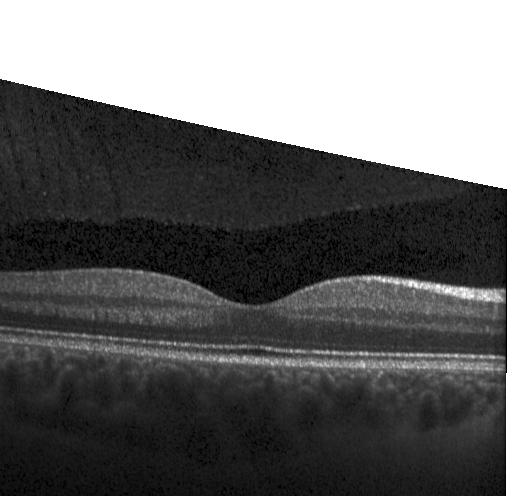

Fovea-centered. OCT B-scan. SD-OCT. Heidelberg Spectralis
Dx: no evidence of choroidal neovascularization, diabetic macular edema, or drusen.